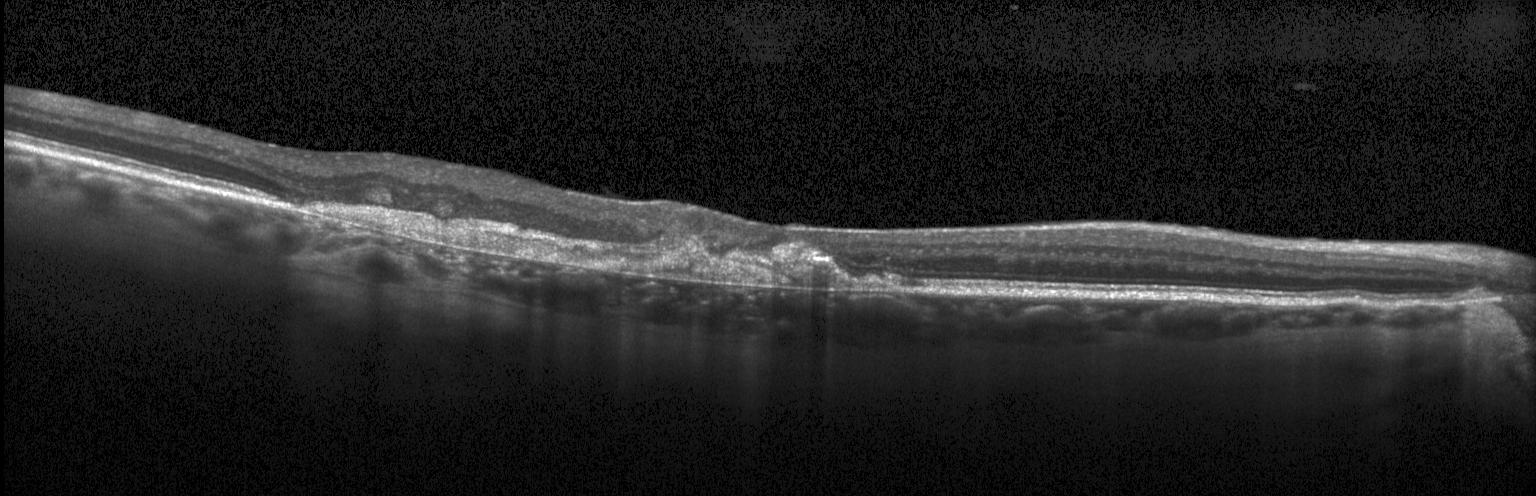 Heidelberg Spectralis · optical coherence tomography scan · SD-OCT · centered on the fovea.
OCT finding: a choroidal neovascular membrane.